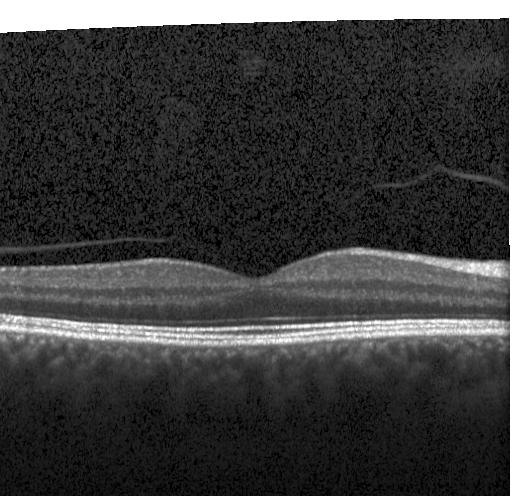 OCT scan showing neither choroidal neovascularization, diabetic macular edema, nor drusen.